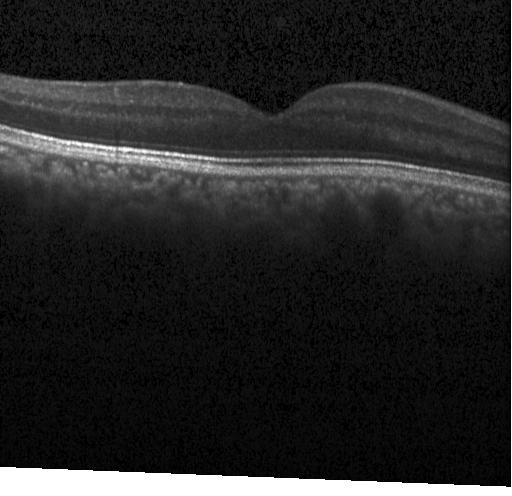 Fovea-centered · OCT B-scan.
Finding: no CNV, no DME, and no drusen.